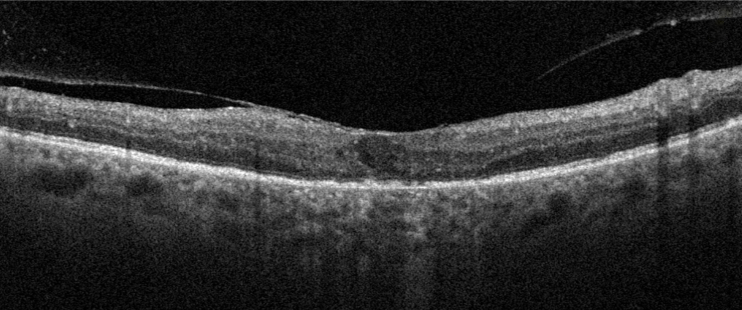

Retinal OCT B-scan. Optovue Avanti RTVue XR.
Impression: diabetic macular edema (DME).